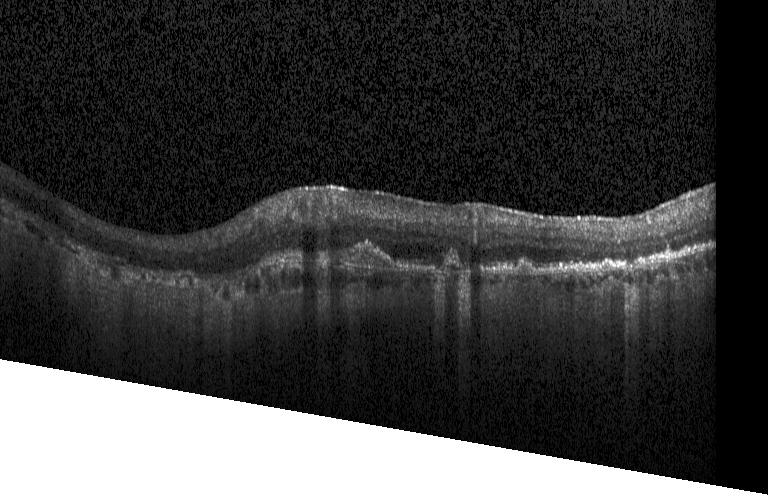 Optical coherence tomography B-scan
Assessment: choroidal neovascularization (CNV).